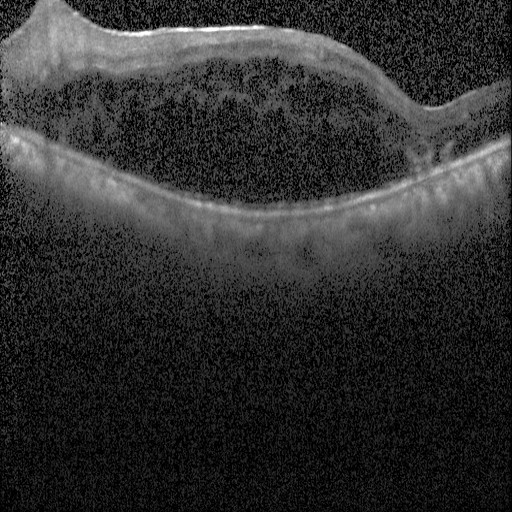 Through the macula. Optical coherence tomography B-scan. Heidelberg Spectralis OCT system. SD-OCT.
Impression: diabetic macular edema.